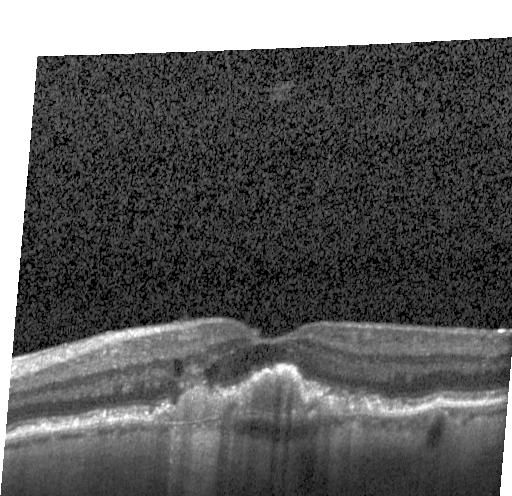
Assessment: CNV.